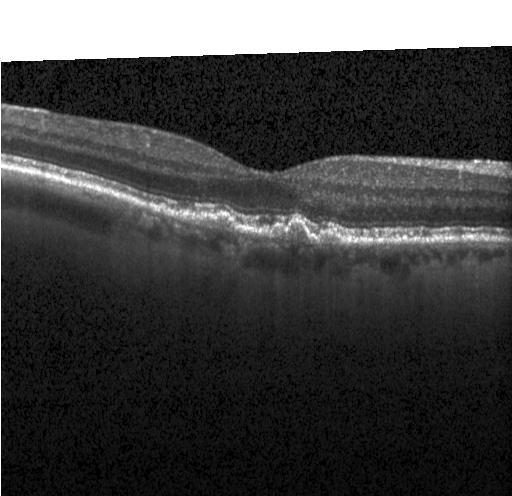

Through the macula · spectral-domain optical coherence tomography · OCT B-scan · Heidelberg Spectralis.
Assessment: sub-RPE drusenoid deposits.